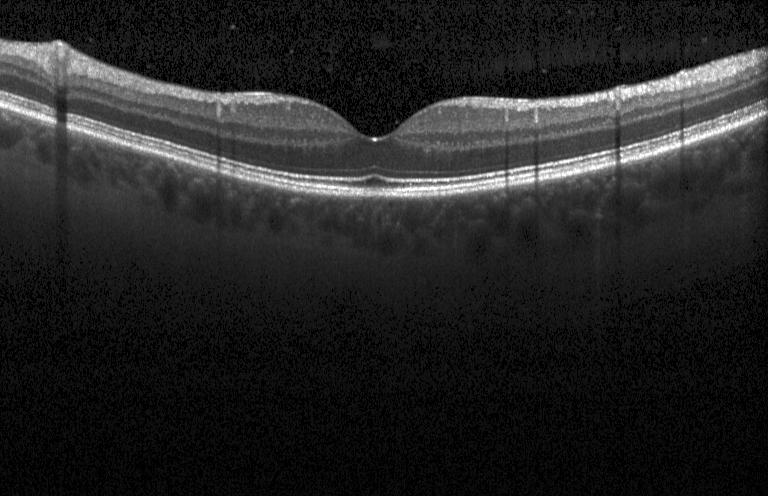
Spectral-domain OCT · retinal OCT cross-section. Finding: no evidence of CNV, DME, or drusen.